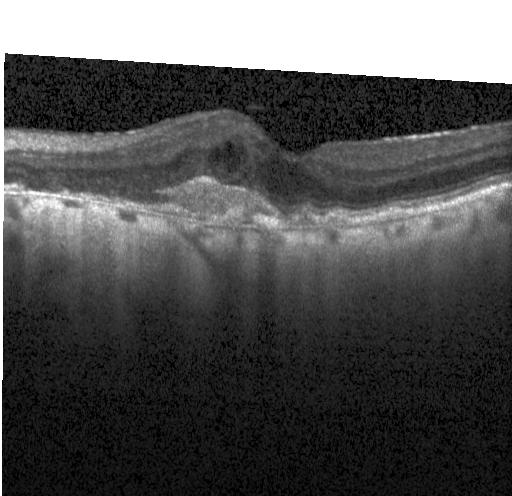

Fovea-centered; optical coherence tomography scan; Heidelberg Spectralis OCT system. The scan shows a choroidal neovascular membrane.